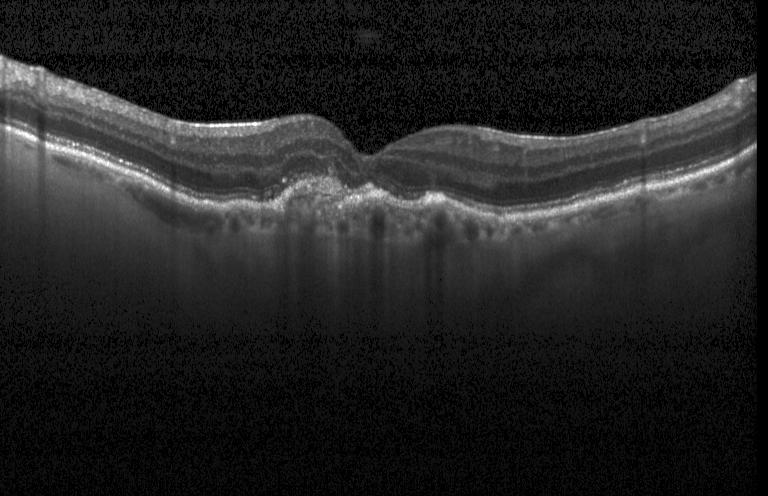
OCT line scan
Diagnosis: CNV.